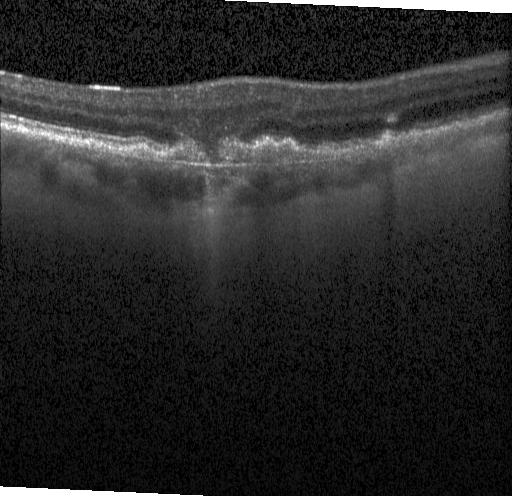

Retinal OCT cross-section showing CNV.